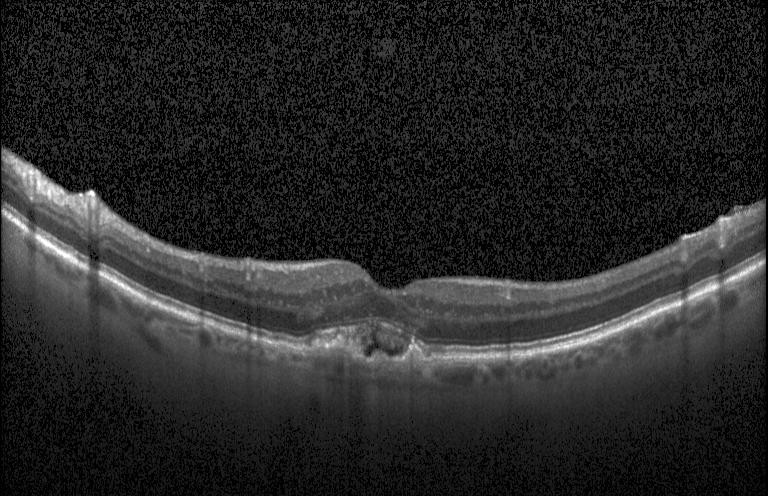

Optical coherence tomography scan, spectral-domain OCT.
Finding: choroidal neovascularization (CNV).